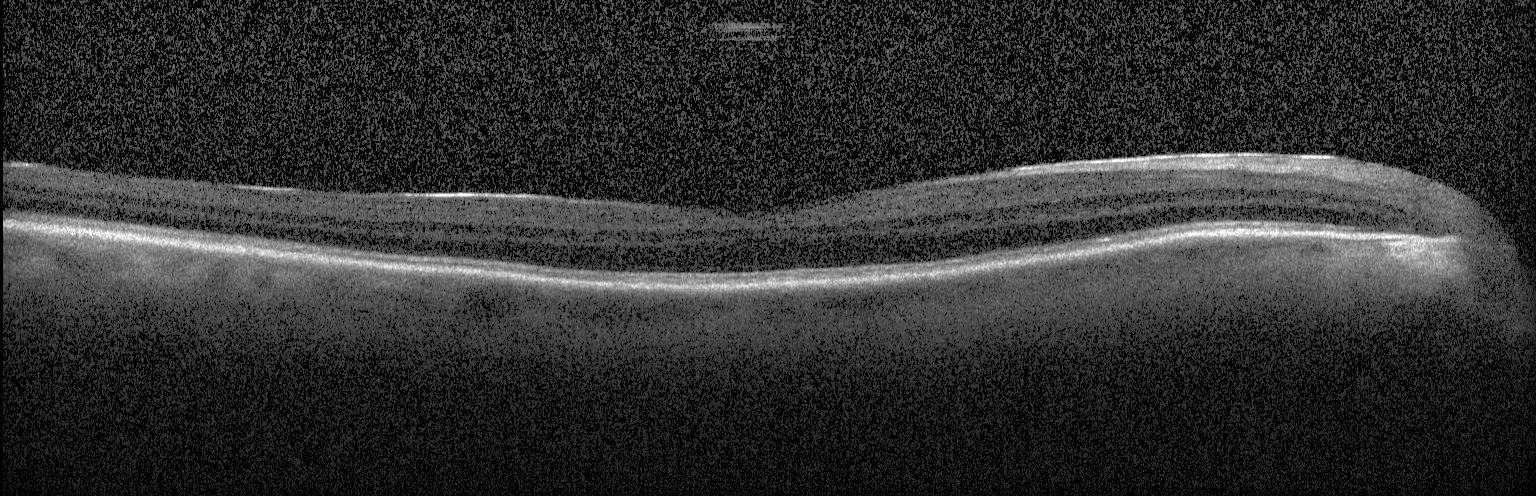

OCT line scan · spectral-domain optical coherence tomography · through the macula — Assessment: no evidence of CNV, DME, or drusen.